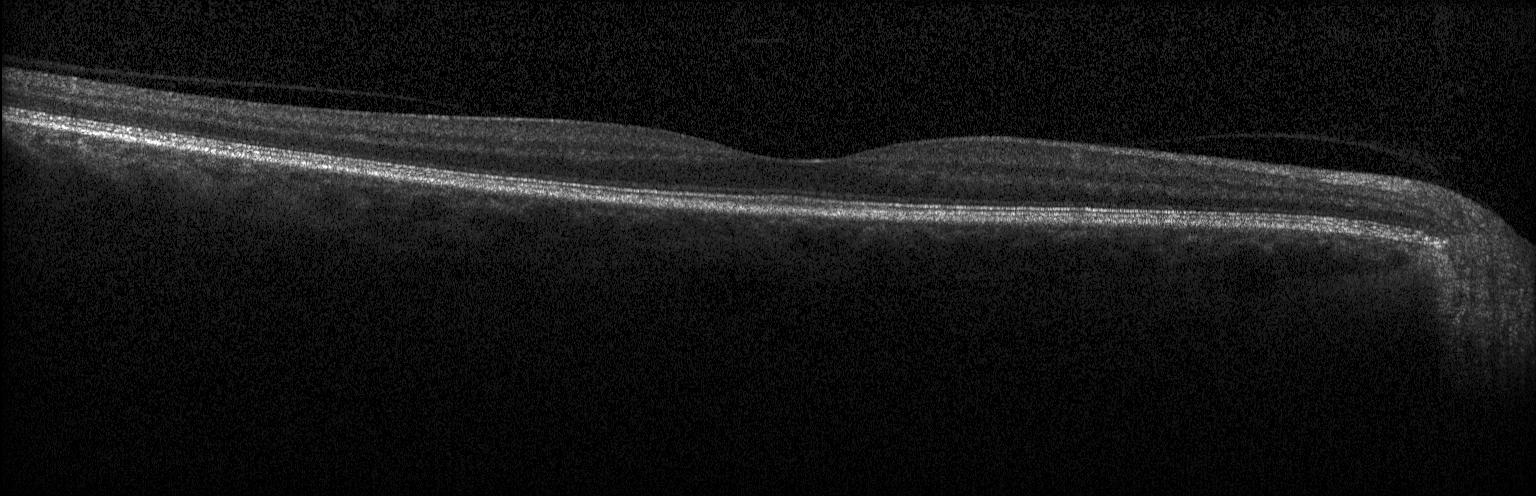

Diagnosis: no CNV, DME, or drusen.